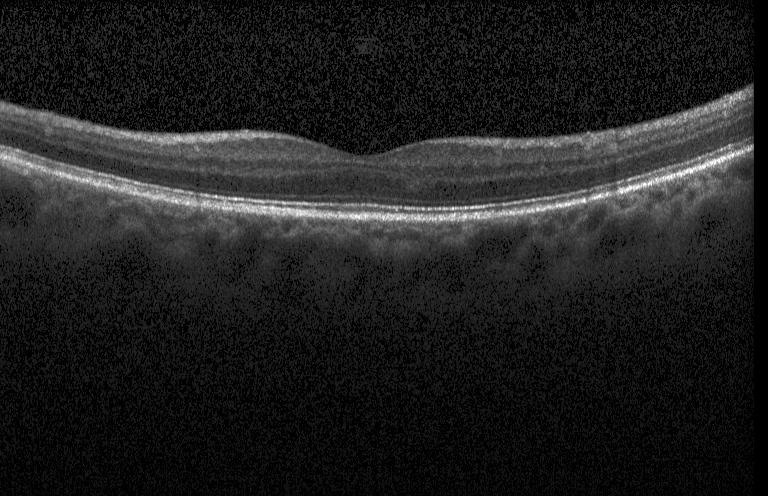

Macular scan. OCT line scan. This B-scan demonstrates neither choroidal neovascularization, diabetic macular edema, nor drusen.